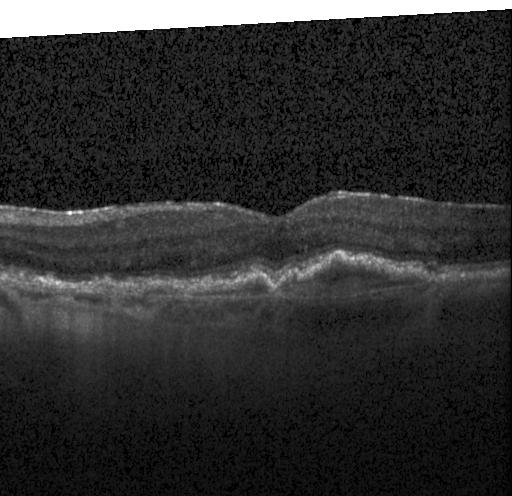
Diagnosis: CNV.